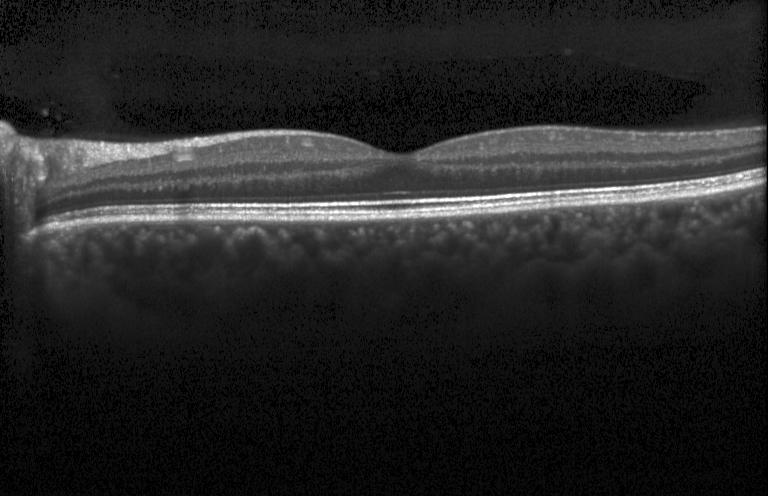

Dx: no choroidal neovascularization, diabetic macular edema, or drusen.